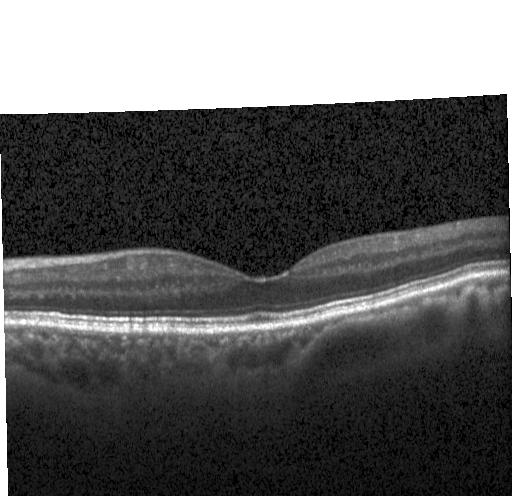
OCT B-scan — Impression: neither CNV, DME, nor drusen.